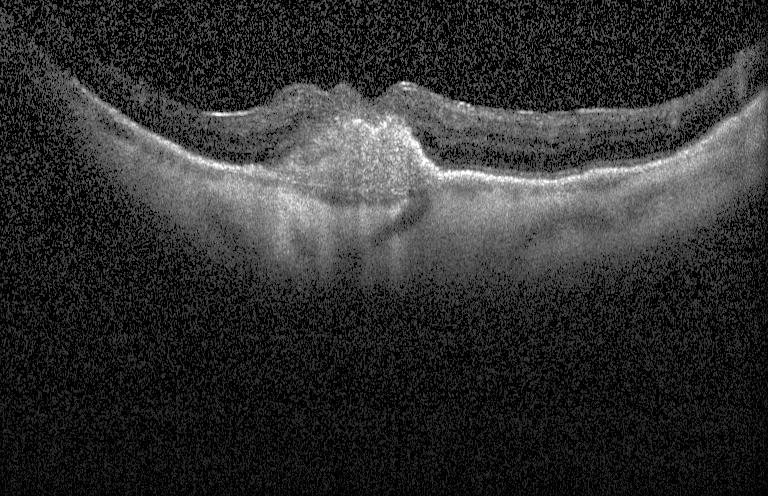 Spectral-domain optical coherence tomography · OCT B-scan.
Choroidal neovascularization.